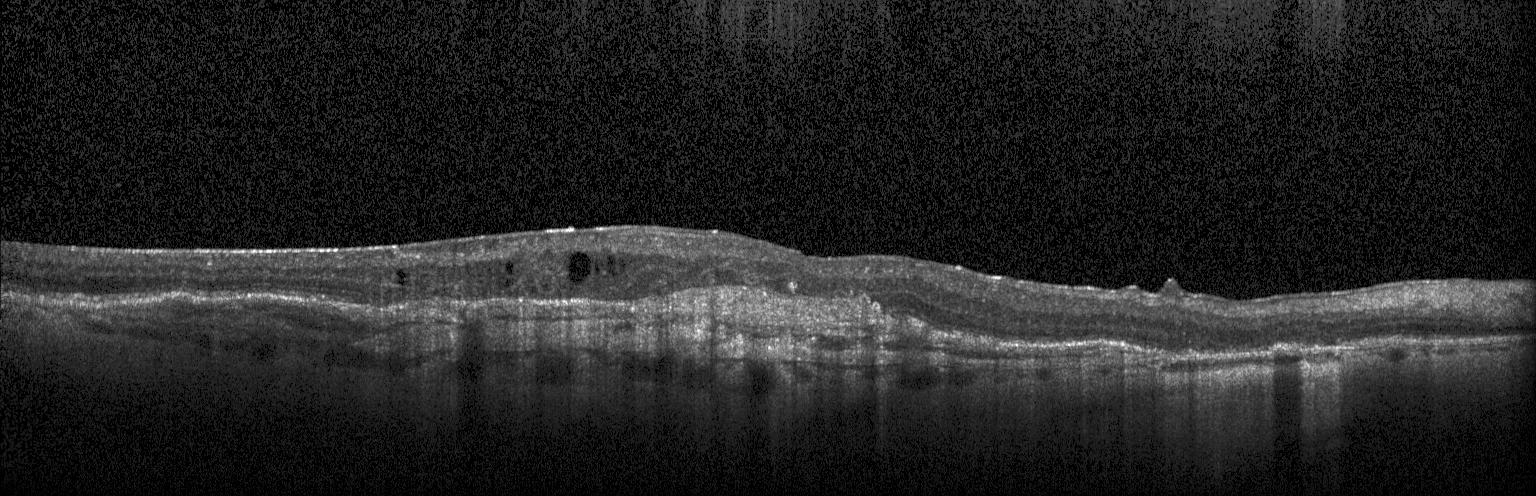 Finding: a choroidal neovascular membrane.